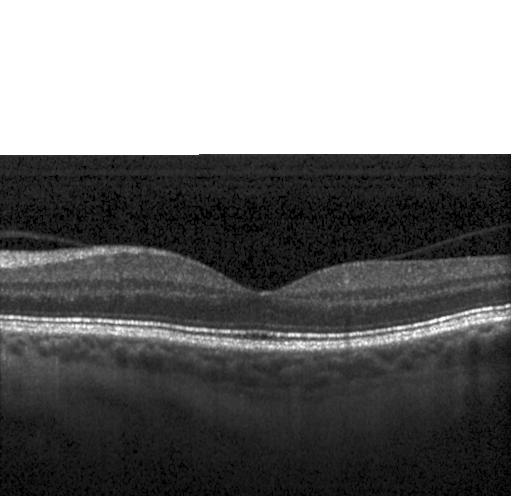 Retinal OCT cross-section showing neither CNV, DME, nor drusen.